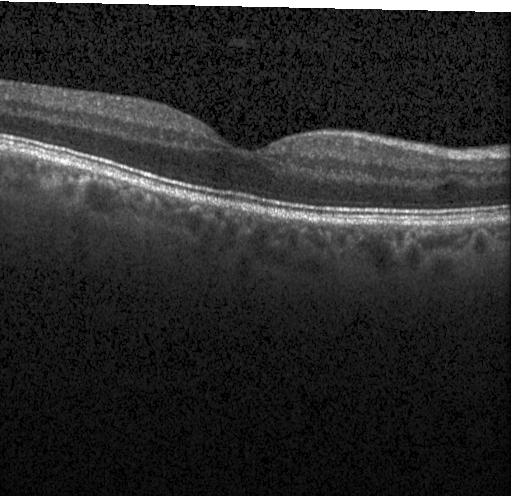
OCT scan showing no choroidal neovascularization, no diabetic macular edema, and no drusen.